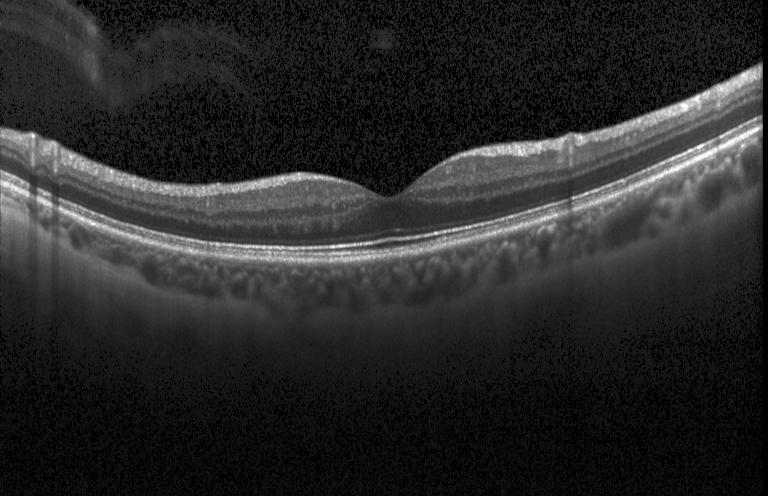

Optical coherence tomography scan — Finding: neither choroidal neovascularization, diabetic macular edema, nor drusen.